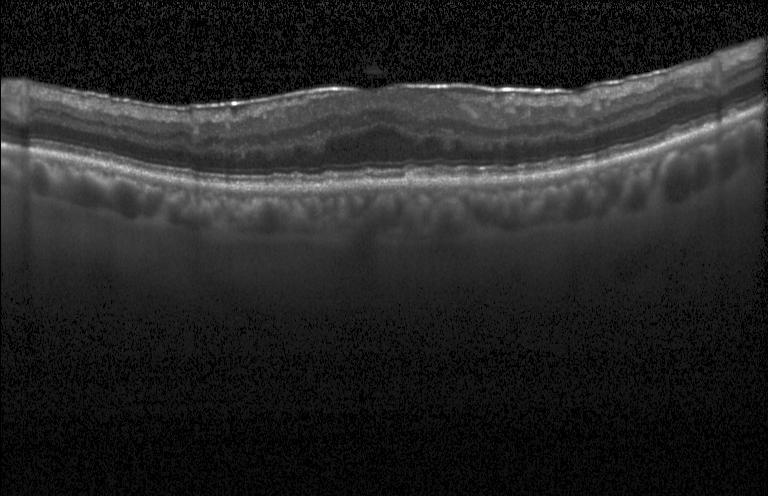 Acquired on a Heidelberg Spectralis. OCT line scan. Diagnosis: drusen.